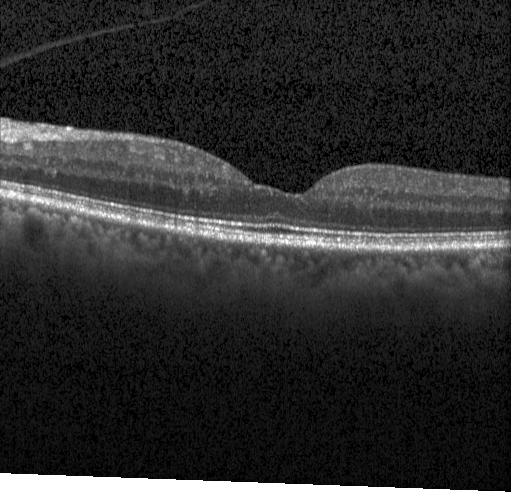 Spectral-domain OCT B-scan: neither choroidal neovascularization, diabetic macular edema, nor drusen.